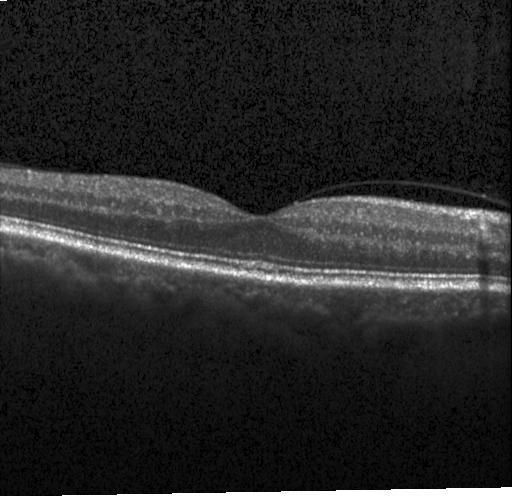

Impression: neither choroidal neovascularization, diabetic macular edema, nor drusen.